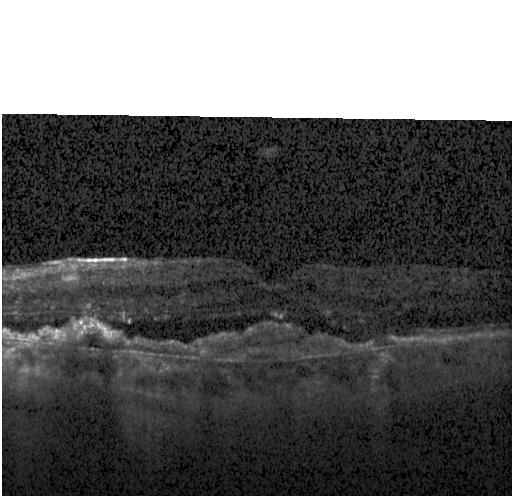

OCT B-scan; Heidelberg Spectralis OCT system; spectral-domain optical coherence tomography
Diagnosis: a choroidal neovascular membrane.